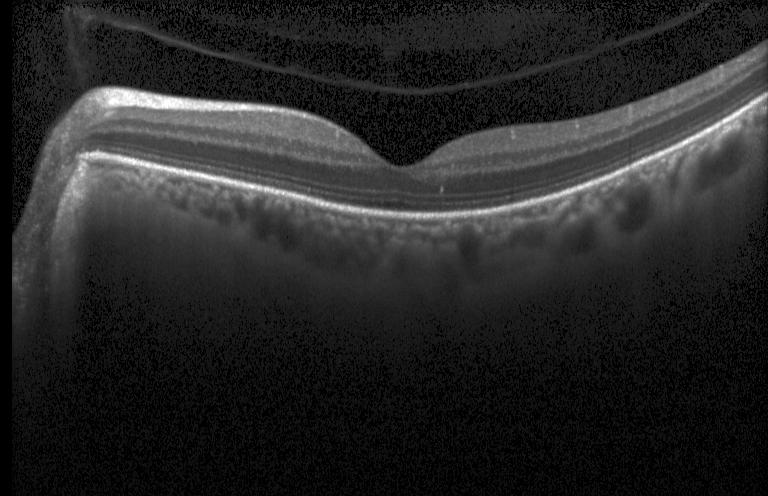
Finding: no choroidal neovascularization, no diabetic macular edema, and no drusen.